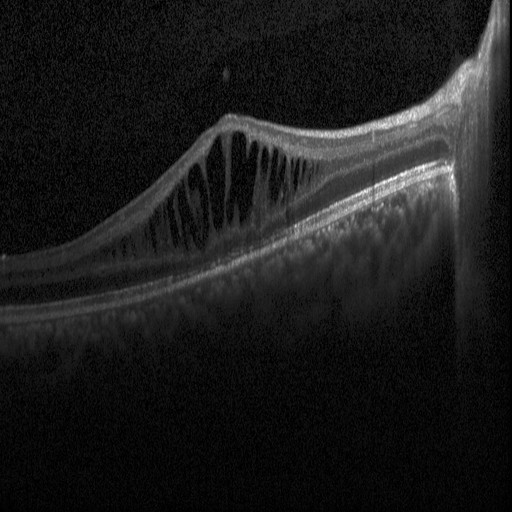
Assessment: DME.